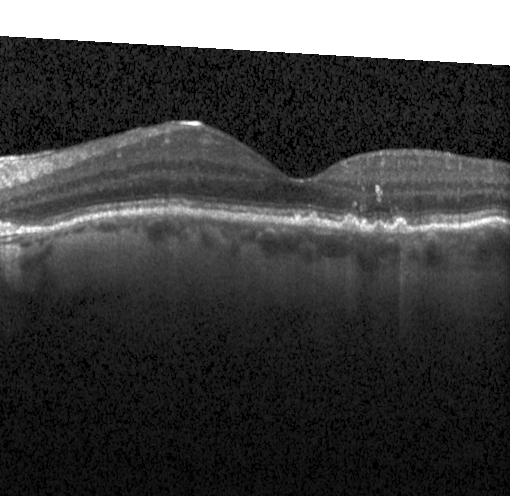 Spectral-domain OCT; optical coherence tomography scan; macular scan — Diagnosis: sub-RPE drusenoid deposits.